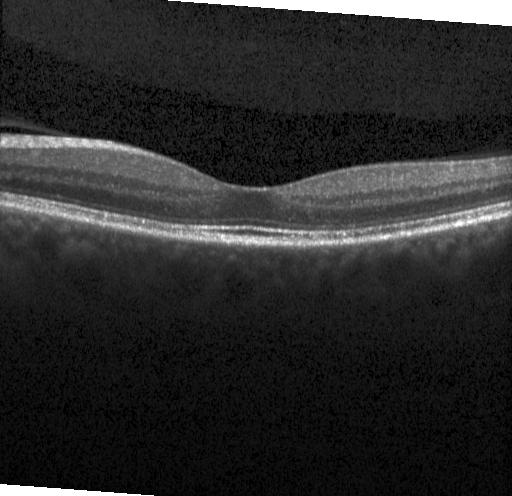 Optical coherence tomography scan; instrument: Heidelberg Spectralis.
The scan shows no evidence of choroidal neovascularization, diabetic macular edema, or drusen.